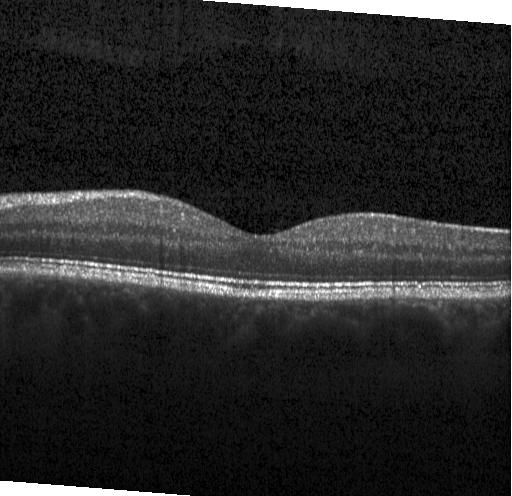

Dx: neither choroidal neovascularization, diabetic macular edema, nor drusen.